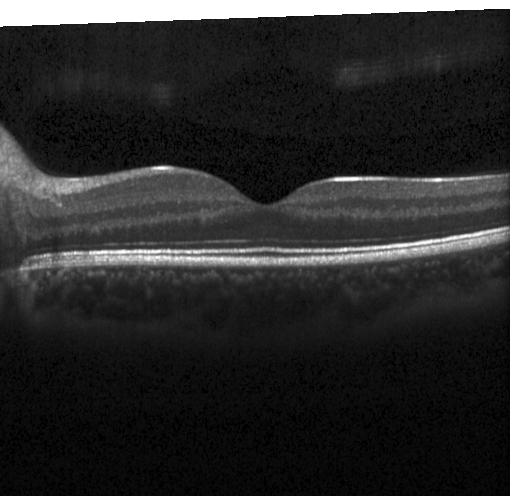

Spectral-domain optical coherence tomography, optical coherence tomography B-scan, macular scan.
Diagnosis: no CNV, no DME, and no drusen.